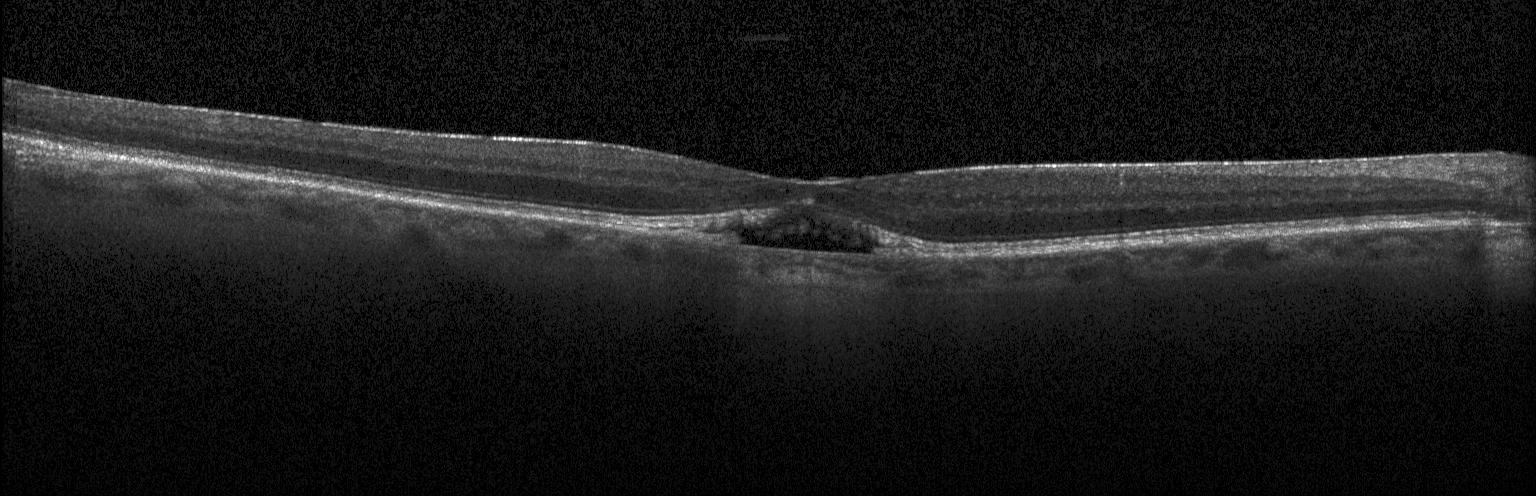 Heidelberg Spectralis OCT system, spectral-domain OCT, optical coherence tomography B-scan — Diagnosis: choroidal neovascularization (CNV).